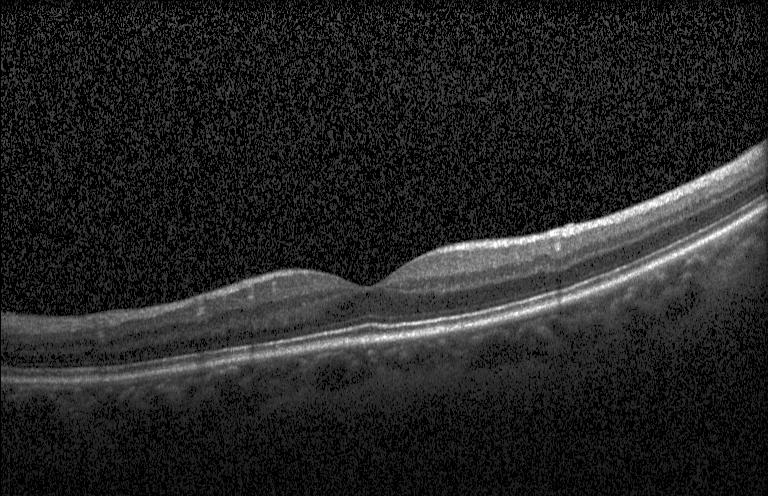

Spectral-domain optical coherence tomography, optical coherence tomography B-scan, horizontal scan through the fovea — Assessment: neither choroidal neovascularization, diabetic macular edema, nor drusen.